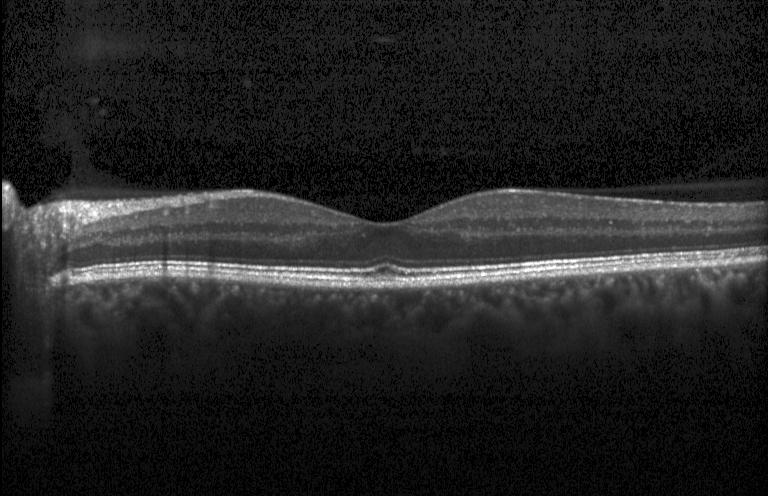
Dx: no choroidal neovascularization, diabetic macular edema, or drusen.